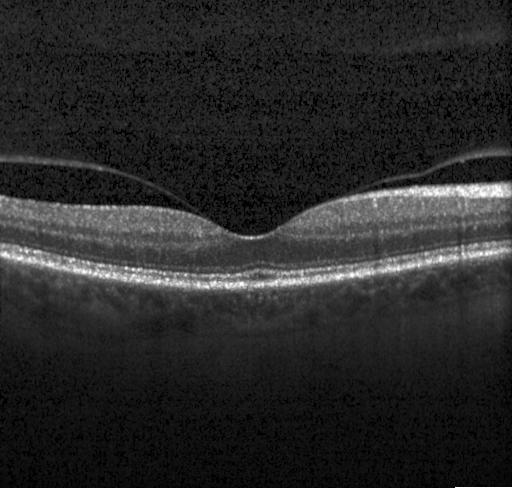

OCT B-scan; spectral-domain OCT.
Finding: no evidence of choroidal neovascularization, diabetic macular edema, or drusen.